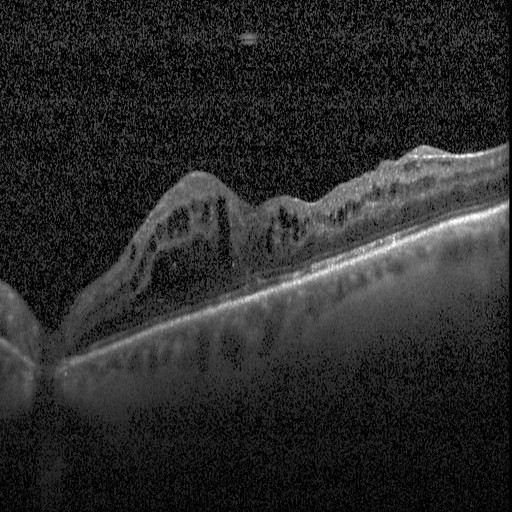 Retinal OCT cross-section — Diagnosis: diabetic macular edema.